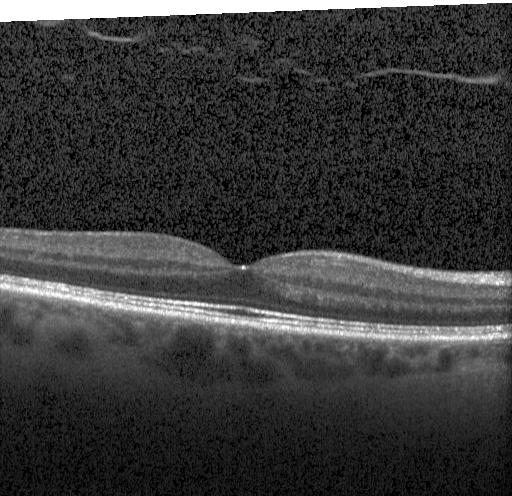
Heidelberg Spectralis; retinal OCT B-scan; centered on the fovea. Finding: neither CNV, DME, nor drusen.